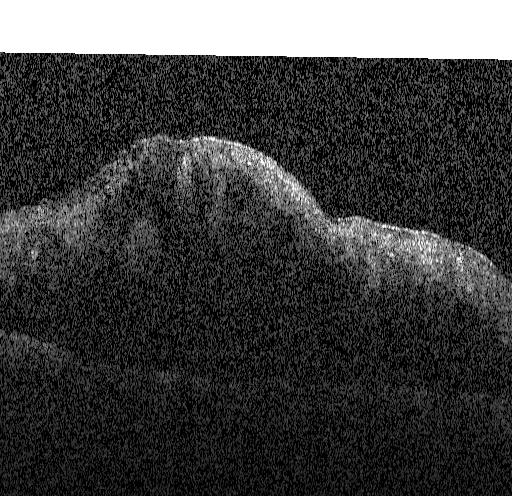

Retinal OCT cross-section. Diagnosis: diabetic macular edema.